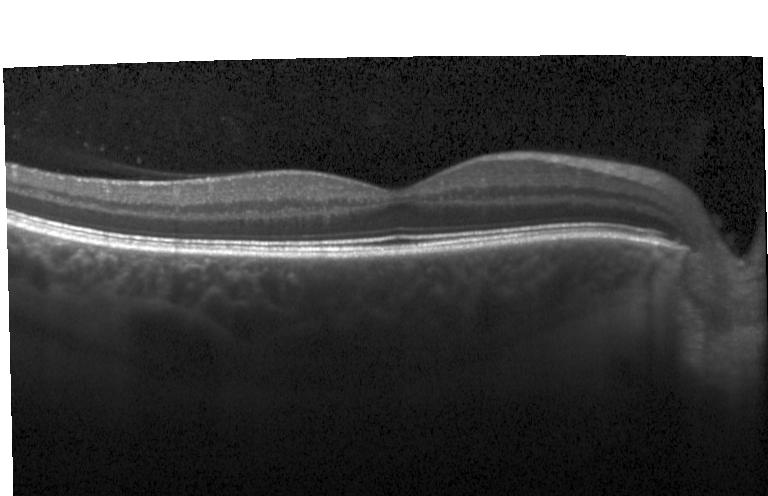 Finding: neither choroidal neovascularization, diabetic macular edema, nor drusen.